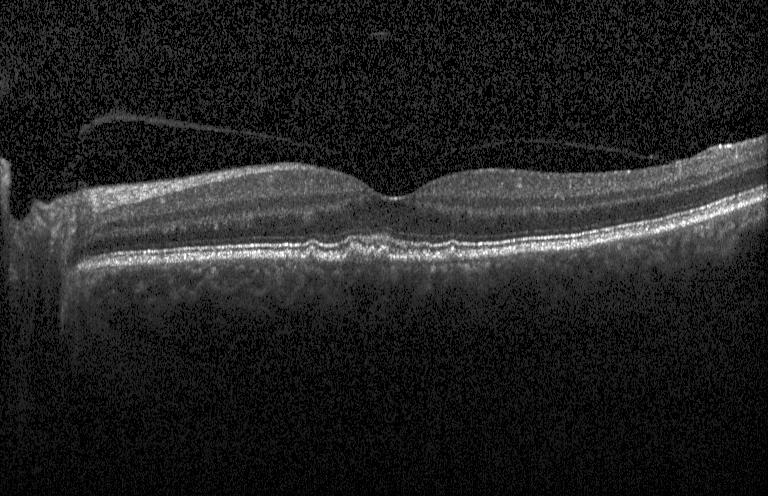
Finding: drusen.